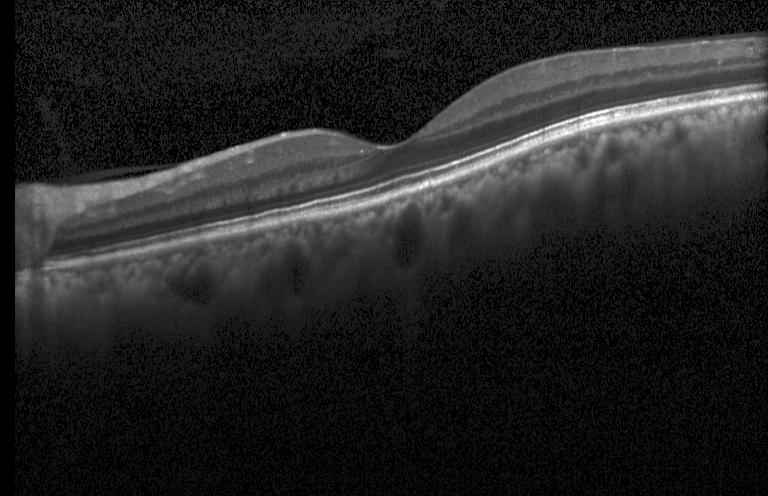

Retinal OCT cross-section · acquired on a Heidelberg Spectralis · SD-OCT.
Dx: no choroidal neovascularization, diabetic macular edema, or drusen.